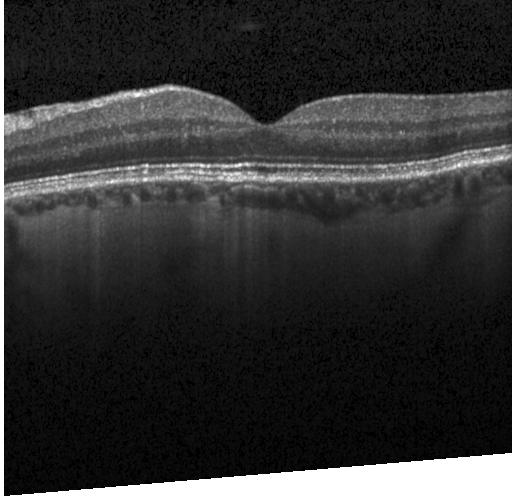
Impression: no choroidal neovascularization, diabetic macular edema, or drusen.